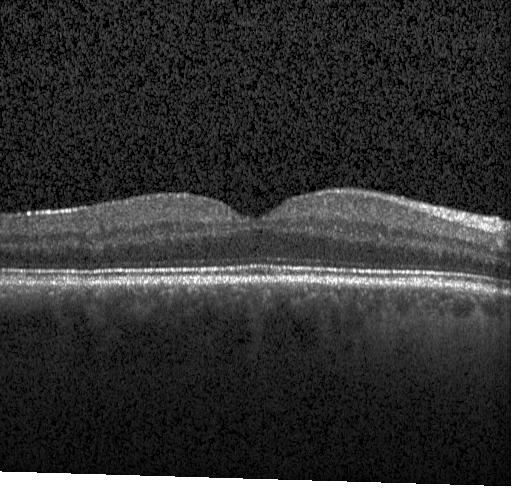 Macular OCT: no choroidal neovascularization, diabetic macular edema, or drusen.